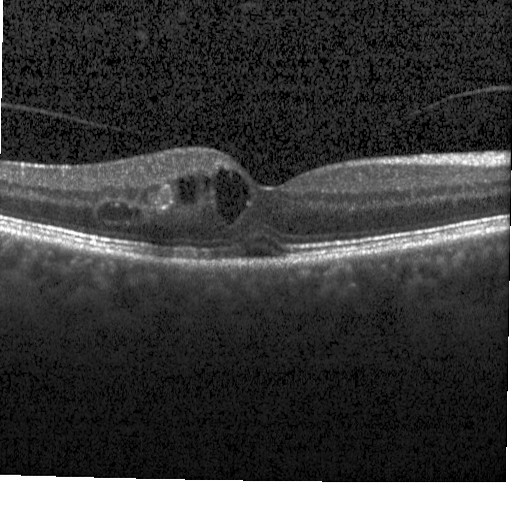 Horizontal scan through the fovea; spectral-domain OCT; OCT line scan. OCT finding: diabetic macular edema.